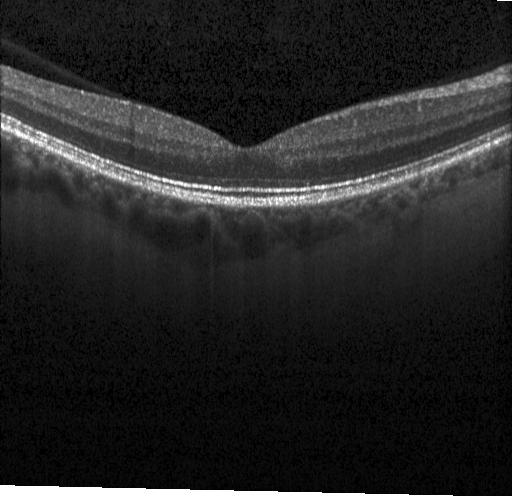

Macular scan, optical coherence tomography B-scan — Assessment: neither CNV, DME, nor drusen.